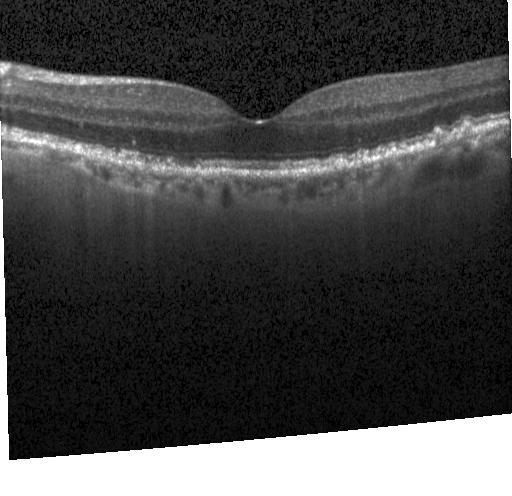 OCT B-scan showing multiple drusen.